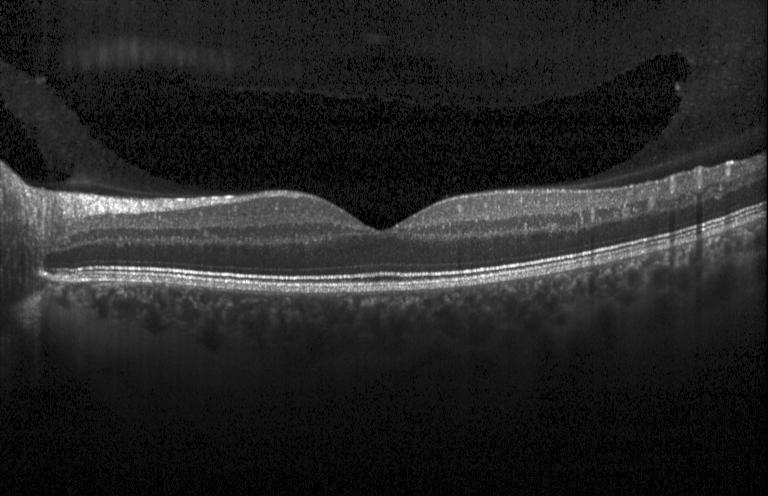 Retinal OCT cross-section, instrument: Heidelberg Spectralis
Finding: no choroidal neovascularization, diabetic macular edema, or drusen.